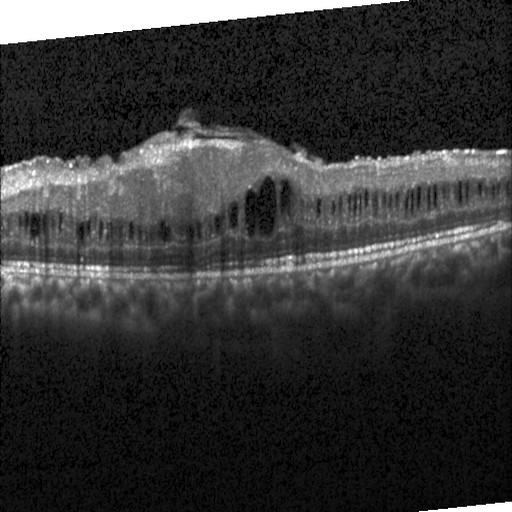
Optical coherence tomography scan. Heidelberg Spectralis. Through the macula. Spectral-domain OCT. Diagnosis: diabetic macular edema (DME).